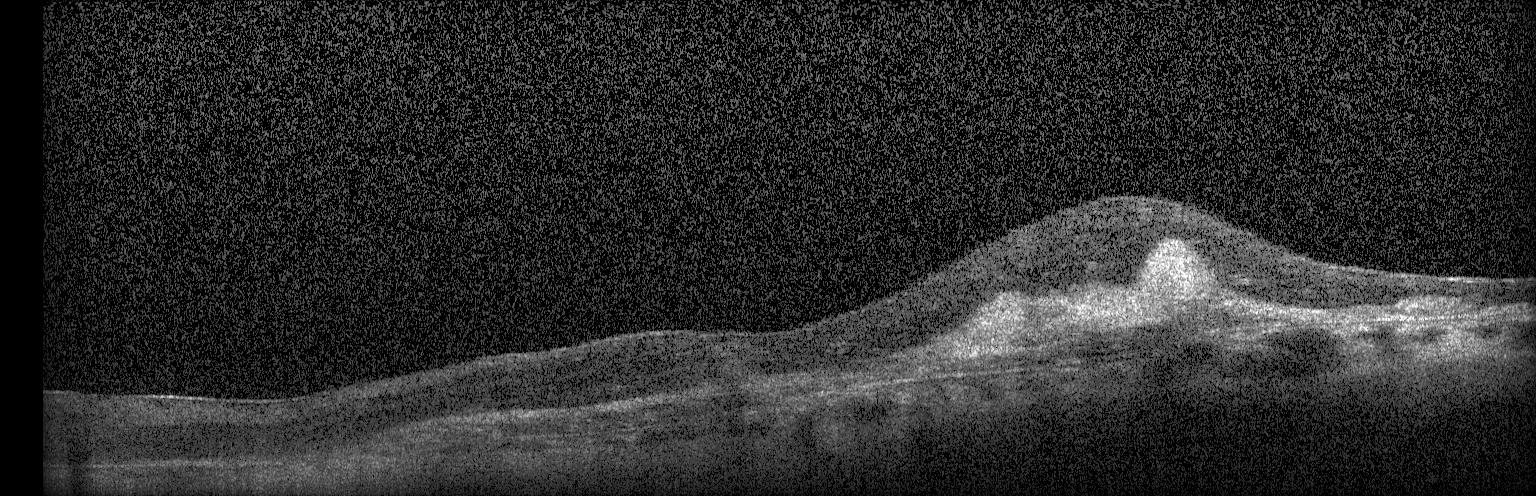 Retinal OCT B-scan. Through the macula. Heidelberg Spectralis. SD-OCT
Dx: choroidal neovascularization.